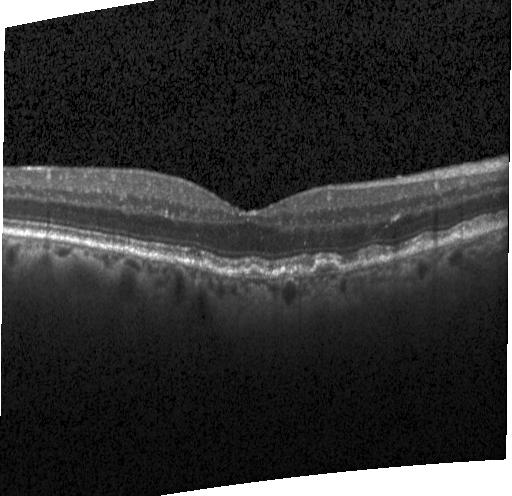 Impression: sub-RPE drusenoid deposits.